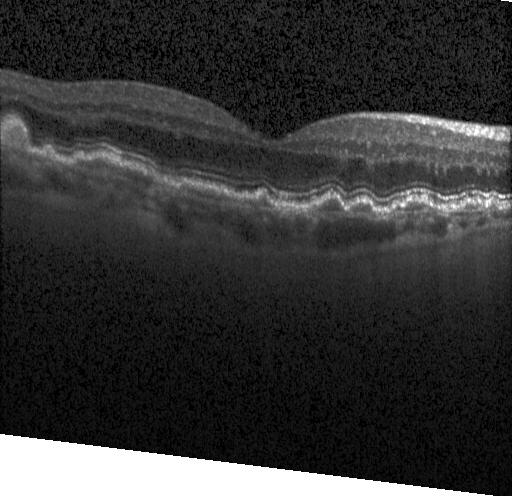
Spectral-domain optical coherence tomography · macular scan · OCT line scan · Heidelberg Spectralis — Dx: drusen.